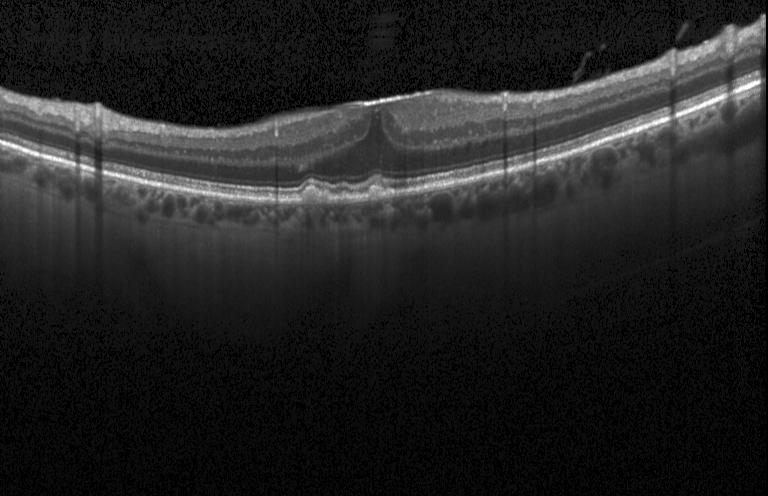
Optical coherence tomography scan.
Assessment: sub-RPE drusenoid deposits.